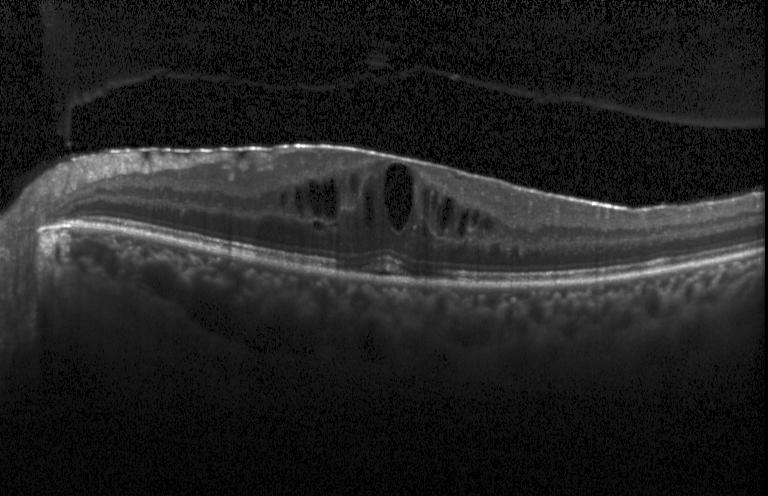

Finding: diabetic macular edema.